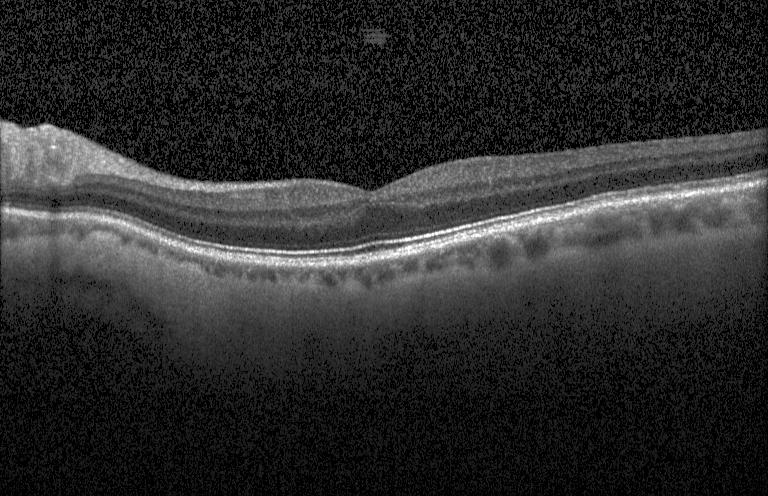
Macular OCT: no evidence of CNV, DME, or drusen.